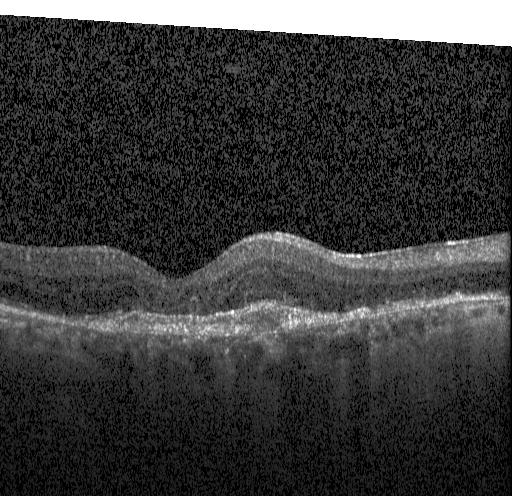 OCT line scan · SD-OCT · instrument: Heidelberg Spectralis · through the macula — Diagnosis: choroidal neovascularization (CNV).